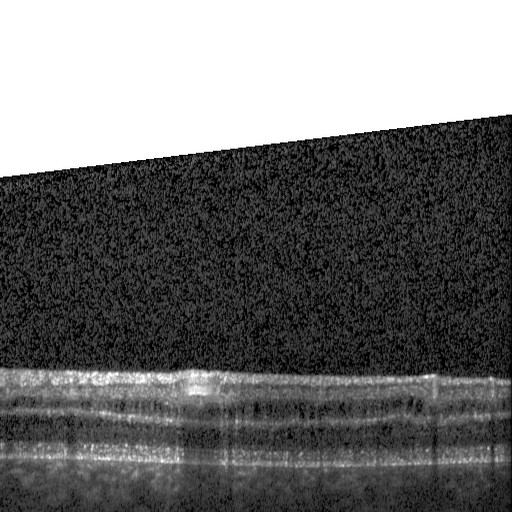
Fovea-centered · optical coherence tomography B-scan
Assessment: diabetic macular edema.